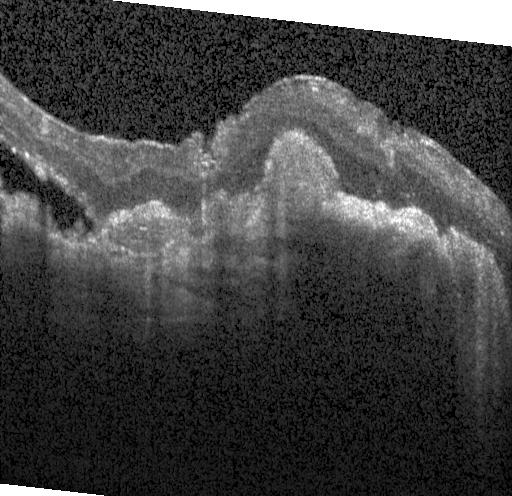
Impression: a choroidal neovascular membrane.